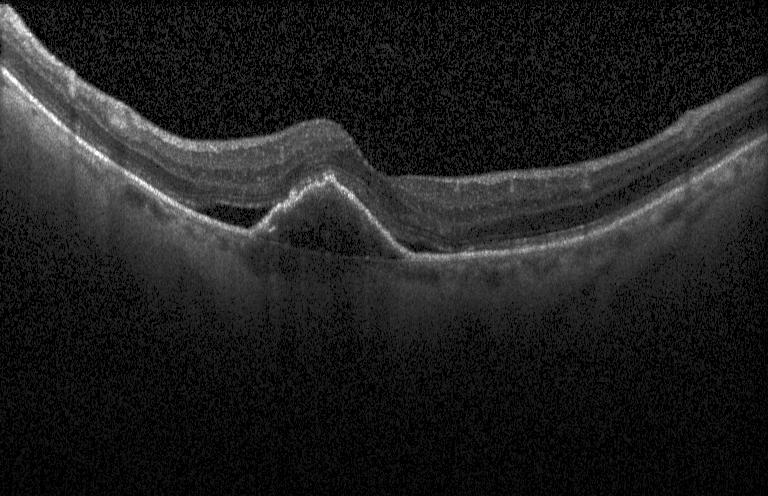
Fovea-centered. Optical coherence tomography scan — Finding: CNV.